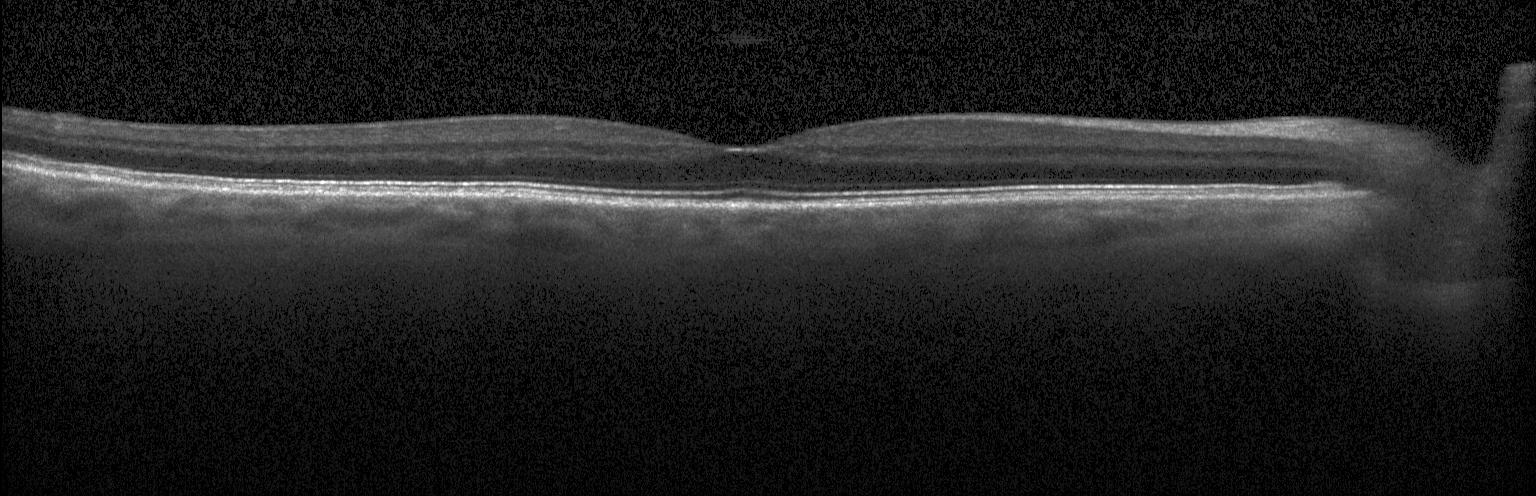

Optical coherence tomography B-scan. Spectral-domain OCT. Heidelberg Spectralis OCT system
Dx: no choroidal neovascularization, no diabetic macular edema, and no drusen.